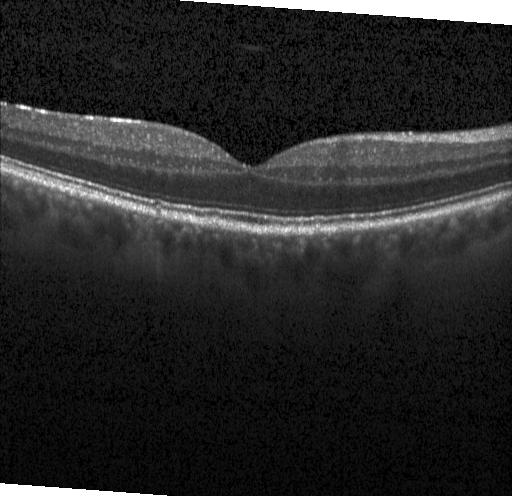
Heidelberg Spectralis OCT system; spectral-domain OCT; optical coherence tomography B-scan
Finding: neither choroidal neovascularization, diabetic macular edema, nor drusen.